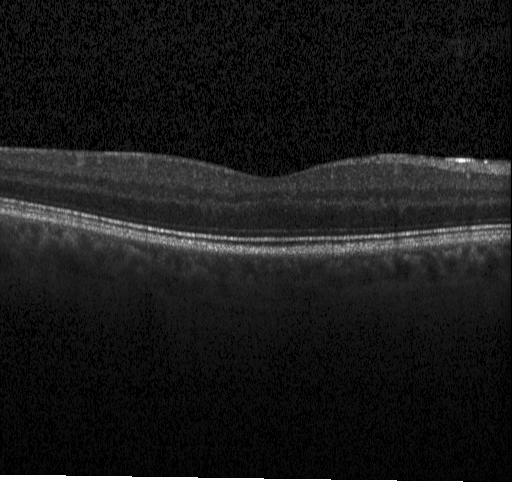
Finding: no CNV, DME, or drusen.